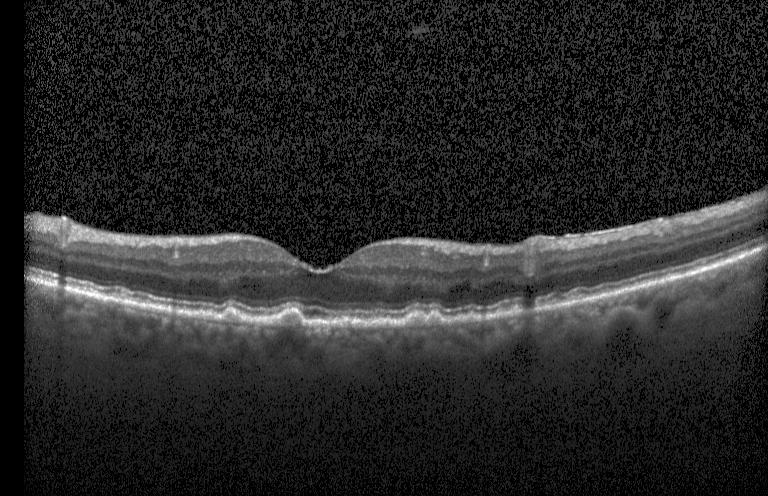

Optical coherence tomography scan · through the macula — This B-scan demonstrates sub-RPE drusenoid deposits.